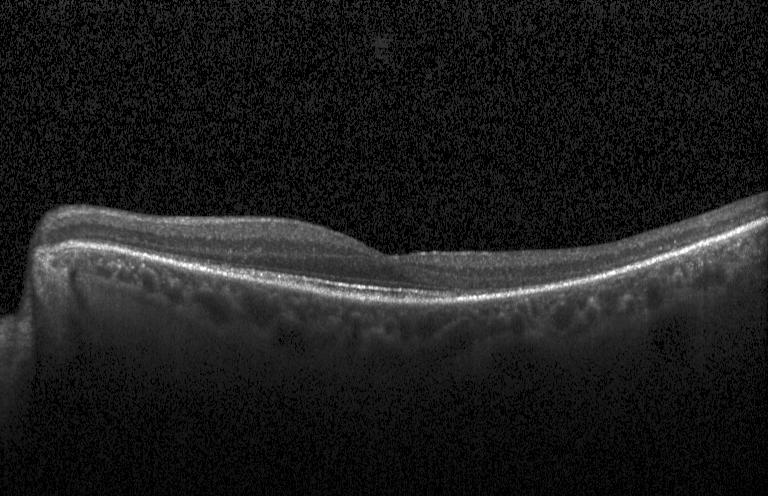
OCT finding: neither CNV, DME, nor drusen.